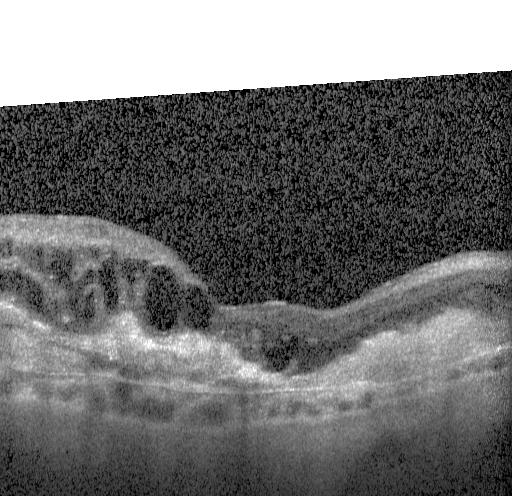
OCT finding: CNV.